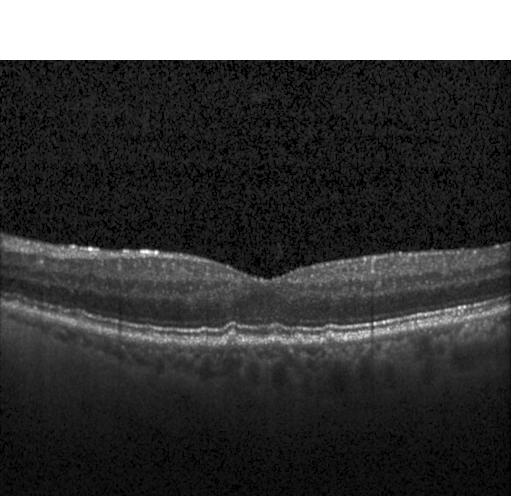
Fovea-centered; retinal OCT cross-section — Sub-RPE drusenoid deposits.